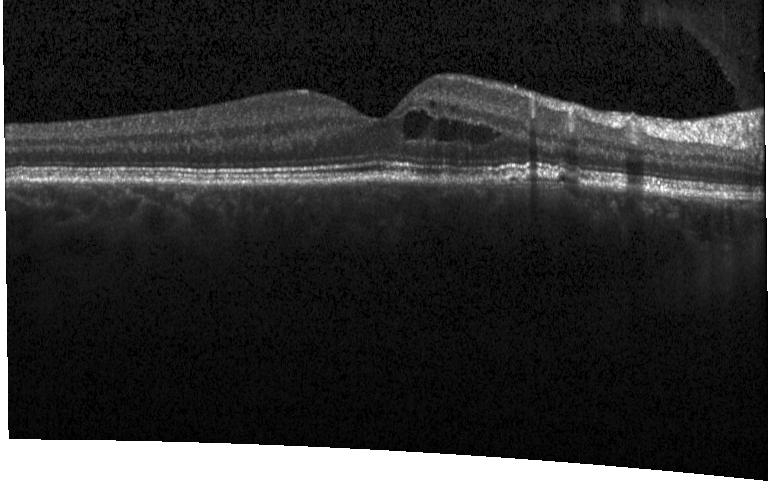

Diagnosis: a choroidal neovascular membrane.